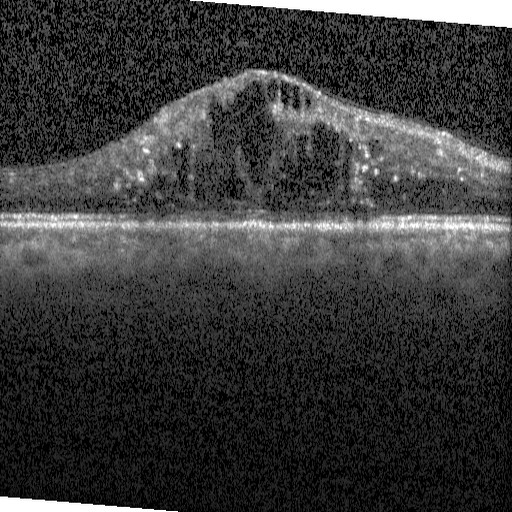 Spectral-domain optical coherence tomography · acquired on a Heidelberg Spectralis · optical coherence tomography B-scan · macular scan — The scan shows DME.